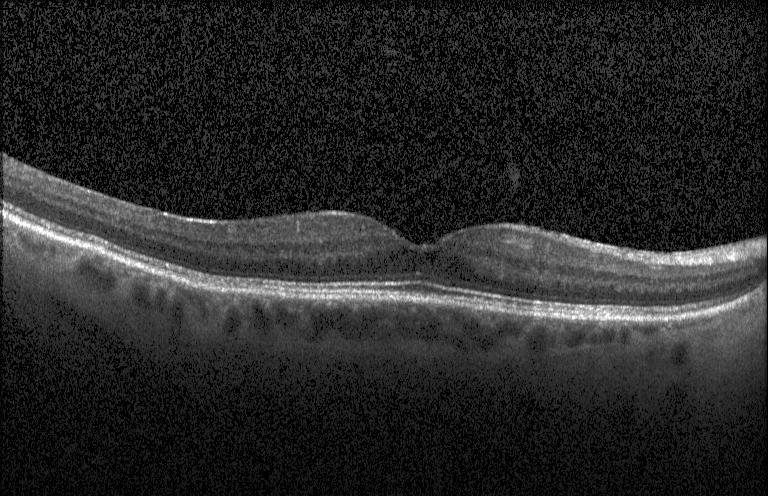

Macular scan, optical coherence tomography scan, Heidelberg Spectralis. Assessment: neither choroidal neovascularization, diabetic macular edema, nor drusen.